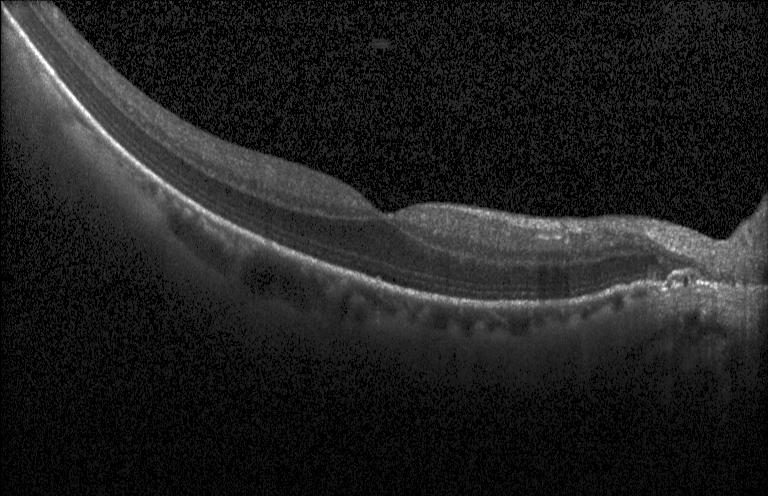 Fovea-centered · OCT B-scan
Finding: no choroidal neovascularization, diabetic macular edema, or drusen.